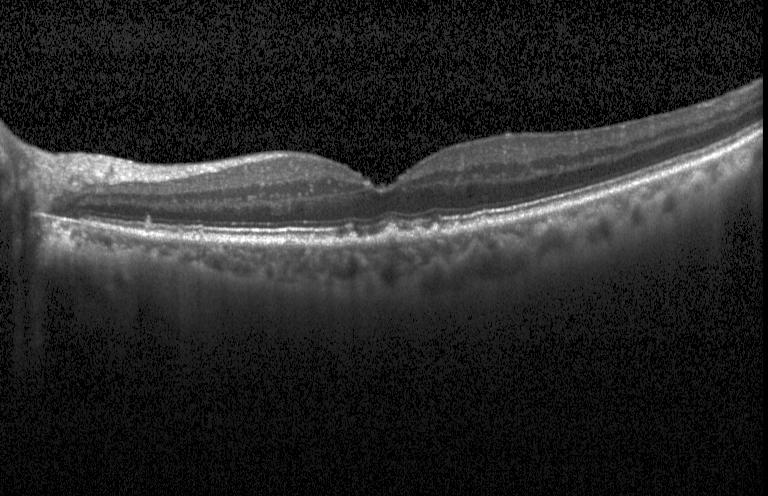

Finding: drusen.